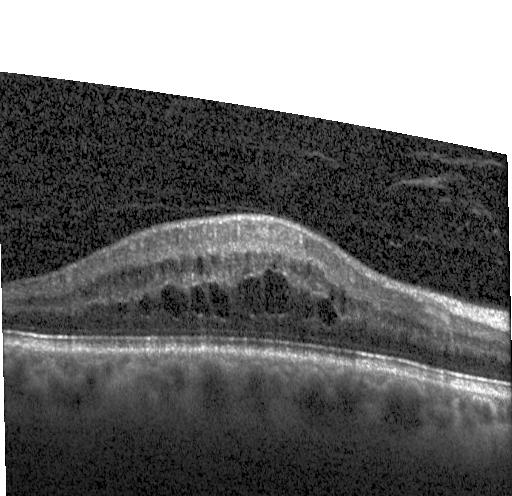
Retinal OCT cross-section · centered on the fovea.
Macular OCT: diabetic macular edema (DME).